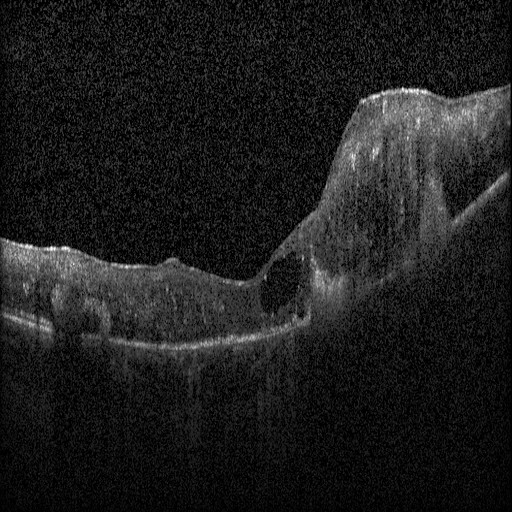 Macular OCT demonstrating diabetic macular edema.